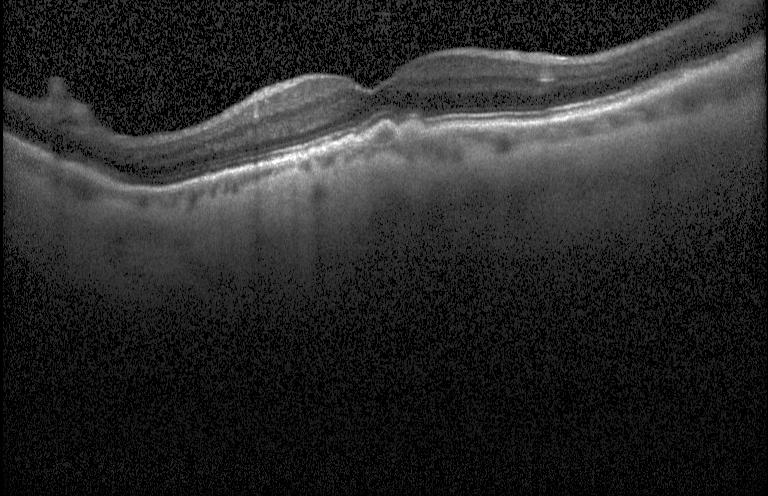 Macular OCT demonstrating multiple drusen.